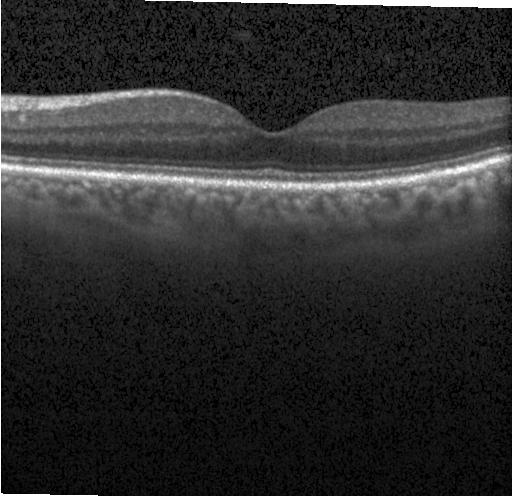 Retinal OCT cross-section showing neither choroidal neovascularization, diabetic macular edema, nor drusen.